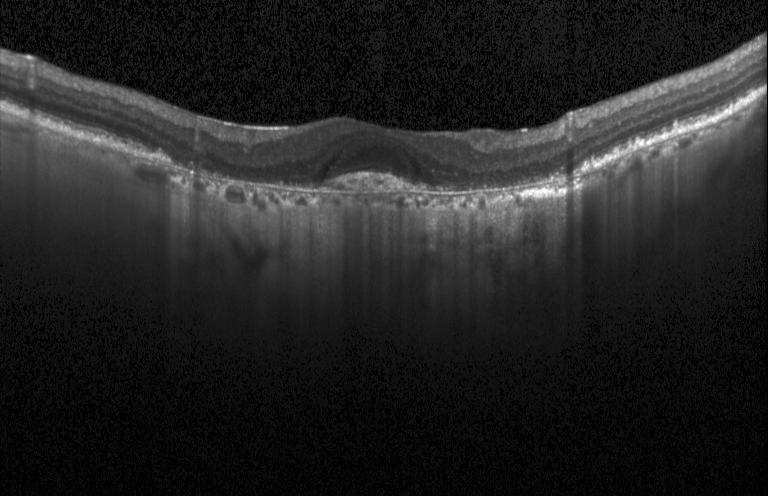

Finding: choroidal neovascularization.